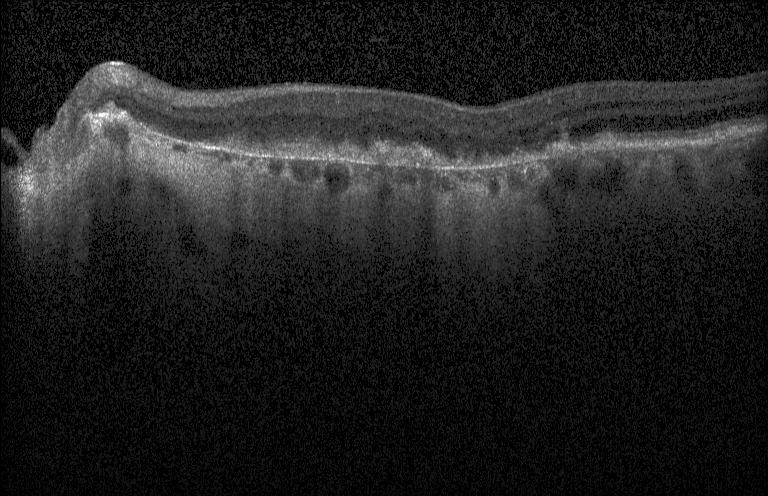
SD-OCT · optical coherence tomography scan
Assessment: choroidal neovascularization.